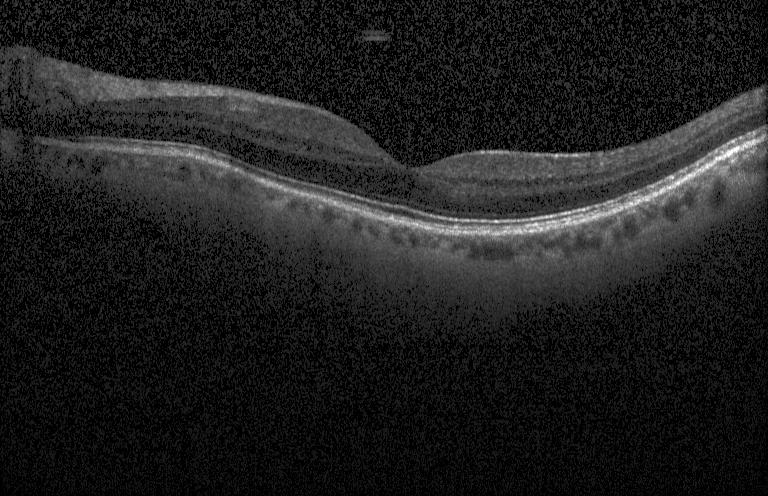
OCT line scan
Diagnosis: no evidence of choroidal neovascularization, diabetic macular edema, or drusen.